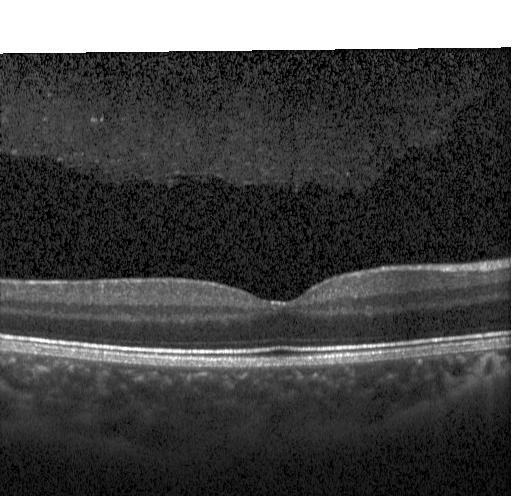 Optical coherence tomography scan, macular scan
Dx: no choroidal neovascularization, no diabetic macular edema, and no drusen.